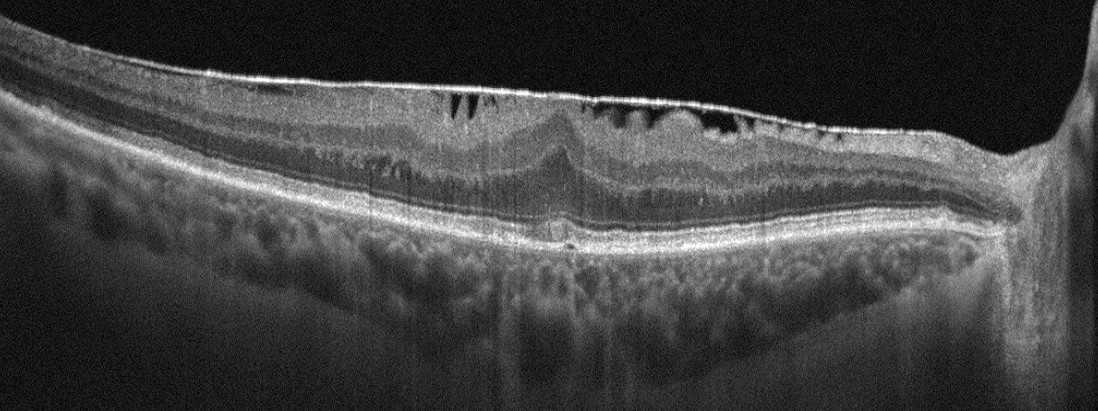
Optovue Avanti RTVue XR · fovea-centered · optical coherence tomography scan
Dx: ERM.